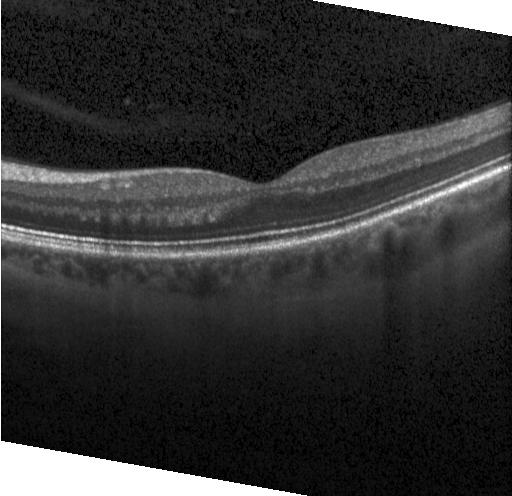 Optical coherence tomography scan — Diagnosis: no choroidal neovascularization, diabetic macular edema, or drusen.